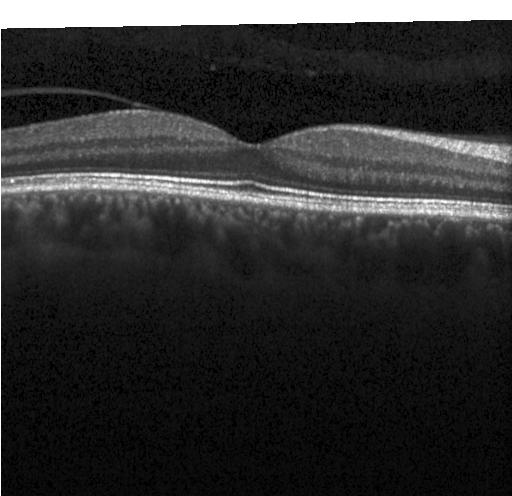
OCT B-scan · fovea-centered
Impression: no choroidal neovascularization, diabetic macular edema, or drusen.